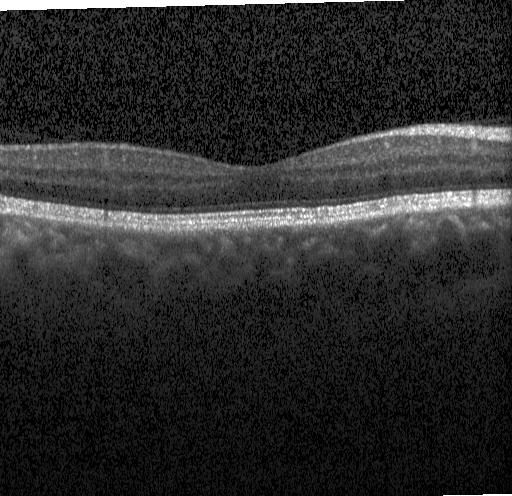
Retinal OCT cross-section, spectral-domain OCT.
No choroidal neovascularization, no diabetic macular edema, and no drusen.